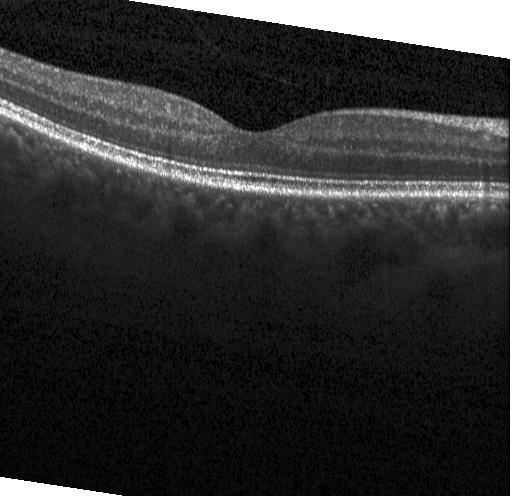 SD-OCT, OCT B-scan, horizontal scan through the fovea, Heidelberg Spectralis — This B-scan demonstrates no choroidal neovascularization, no diabetic macular edema, and no drusen.